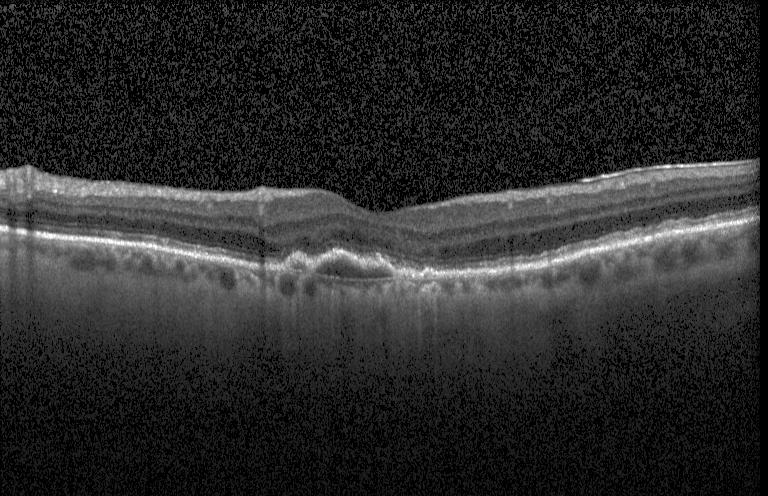

Spectral-domain OCT B-scan: a choroidal neovascular membrane.